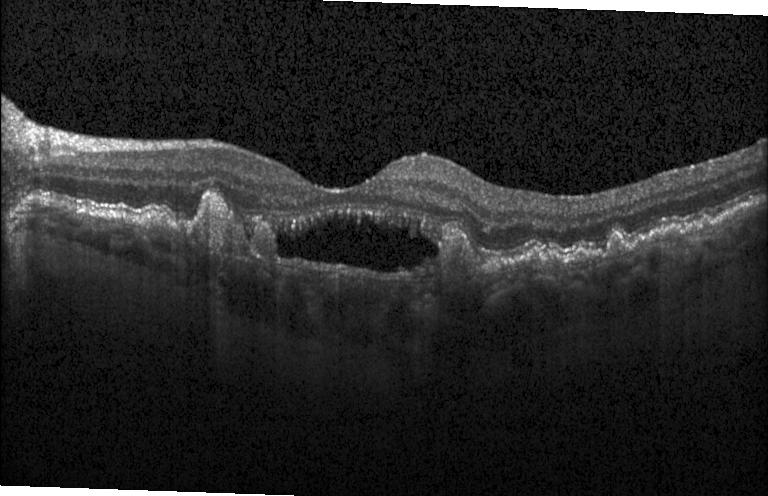

This B-scan demonstrates a choroidal neovascular membrane.